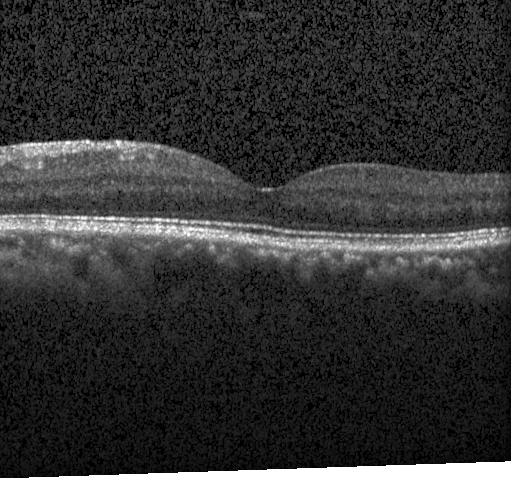
OCT line scan. The scan shows no evidence of choroidal neovascularization, diabetic macular edema, or drusen.